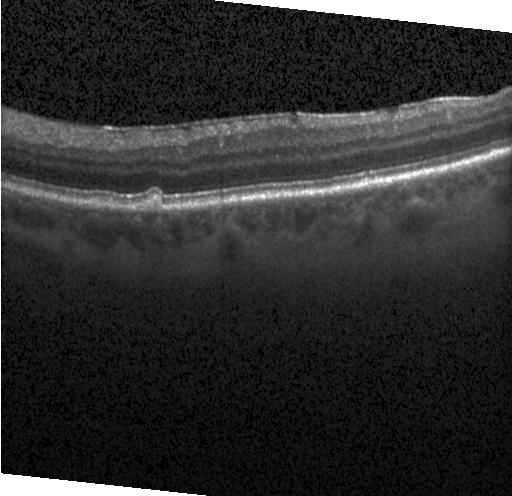 Through the macula, spectral-domain optical coherence tomography, OCT line scan
Diagnosis: drusen.